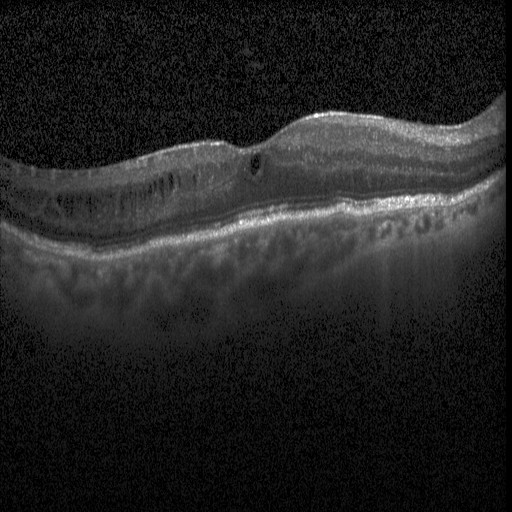 Diagnosis: diabetic macular edema (DME).